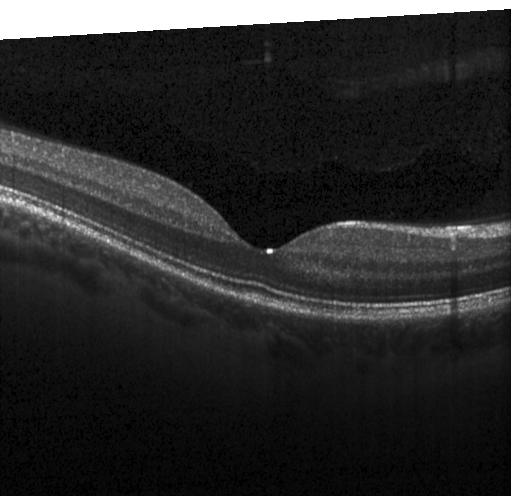
Spectral-domain OCT; retinal OCT B-scan; fovea-centered — Impression: no CNV, no DME, and no drusen.